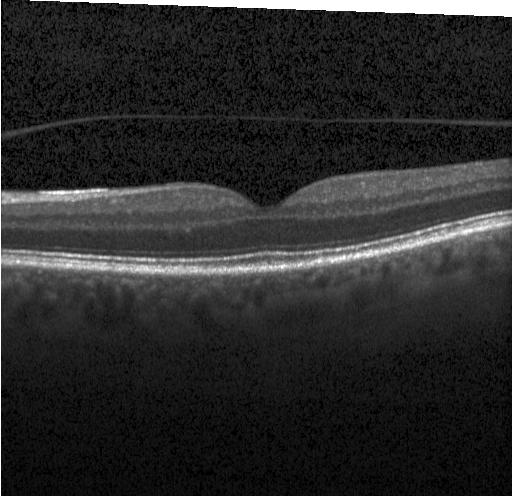
OCT B-scan; Heidelberg Spectralis; horizontal scan through the fovea. Finding: neither CNV, DME, nor drusen.